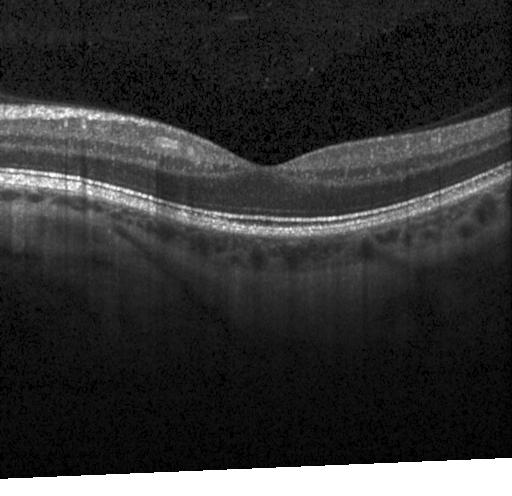
Optical coherence tomography scan. Instrument: Heidelberg Spectralis. Spectral-domain OCT. Macular scan. Dx: no CNV, no DME, and no drusen.